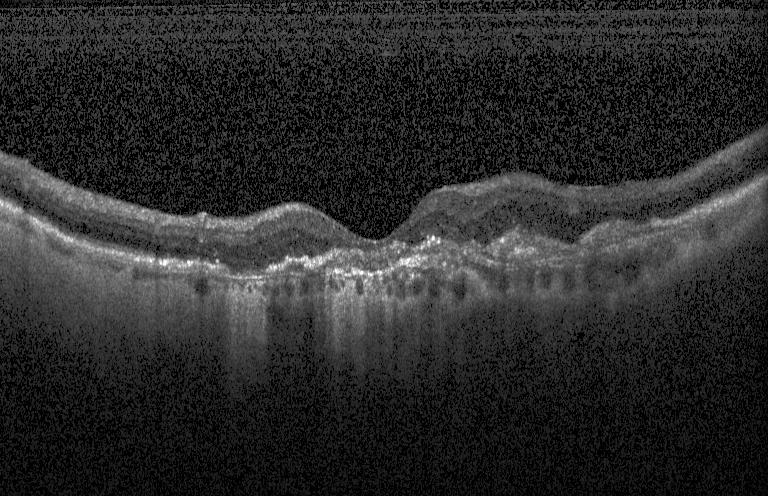

Assessment: a choroidal neovascular membrane.